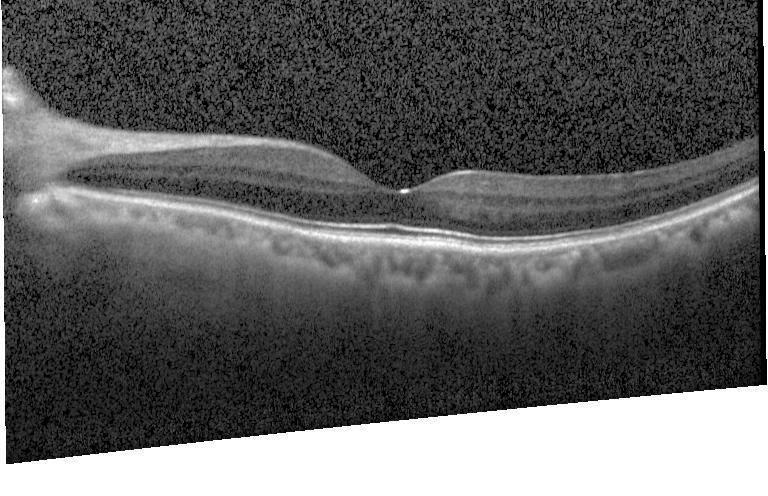
Heidelberg Spectralis OCT system. OCT line scan. Impression: neither choroidal neovascularization, diabetic macular edema, nor drusen.